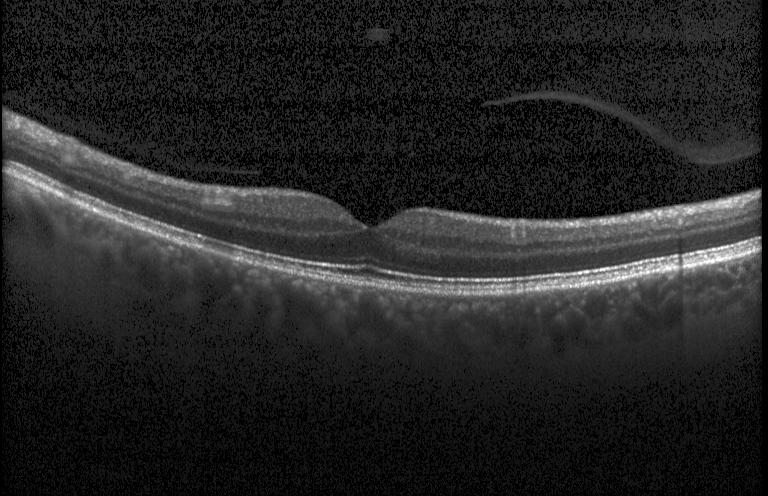 Optical coherence tomography scan · instrument: Heidelberg Spectralis.
Diagnosis: no choroidal neovascularization, diabetic macular edema, or drusen.